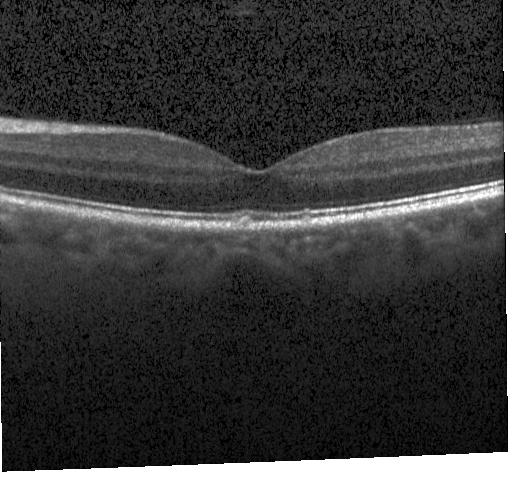 Optical coherence tomography B-scan · SD-OCT · Heidelberg Spectralis OCT system — Diagnosis: sub-RPE drusenoid deposits.